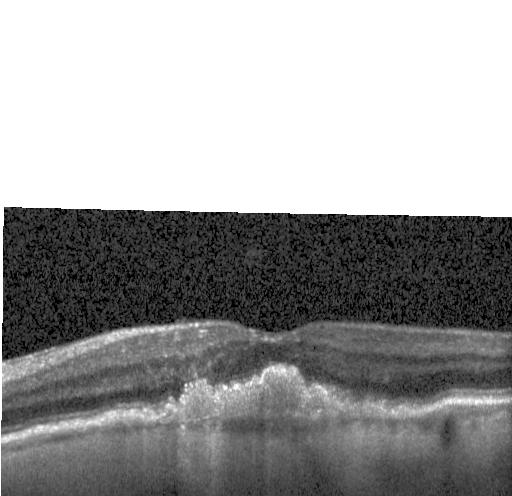 Optical coherence tomography scan — Diagnosis: choroidal neovascularization (CNV).